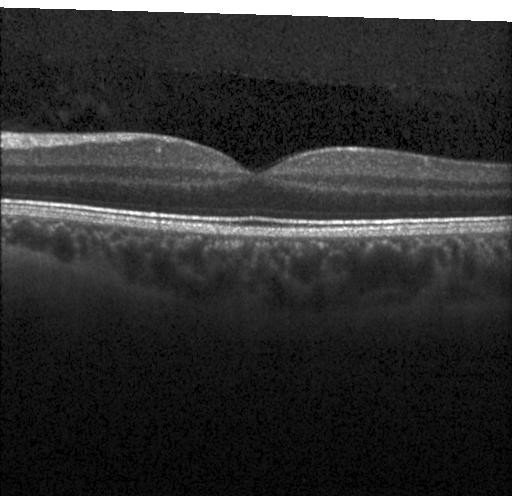 Macular scan, OCT B-scan.
Finding: no CNV, no DME, and no drusen.